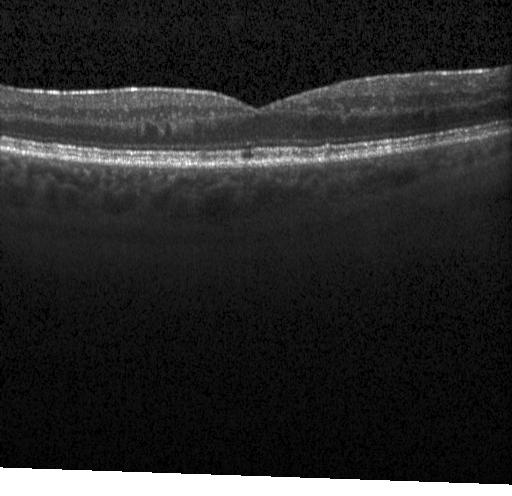 OCT B-scan.
Dx: no CNV, DME, or drusen.